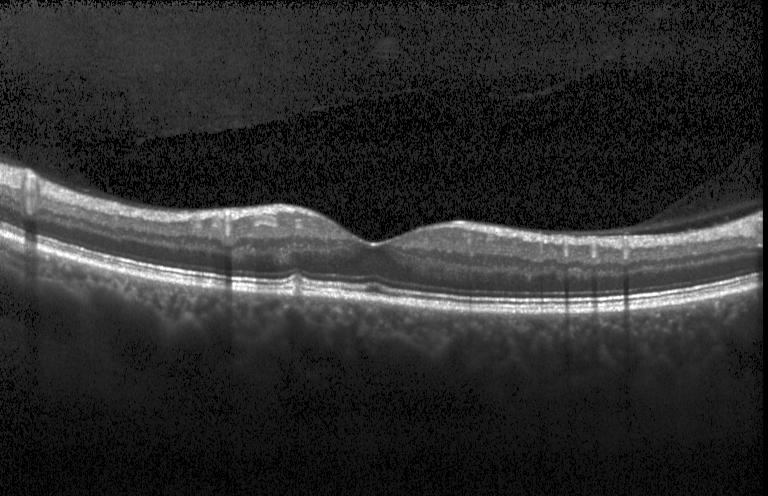

Optical coherence tomography B-scan; acquired on a Heidelberg Spectralis; spectral-domain optical coherence tomography; centered on the fovea. Diagnosis: multiple drusen.